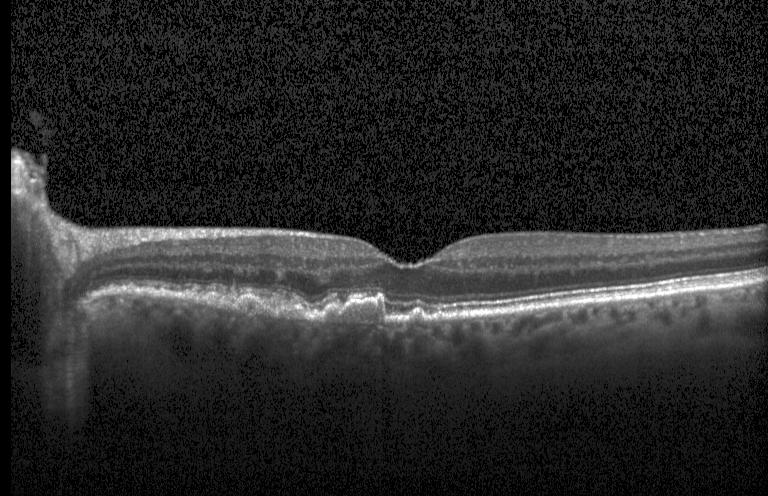
Fovea-centered; optical coherence tomography scan; SD-OCT; instrument: Heidelberg Spectralis. Finding: multiple drusen.